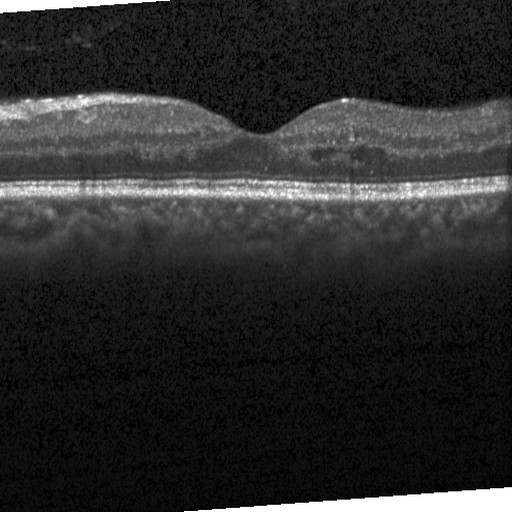
OCT line scan
This B-scan demonstrates diabetic macular edema.